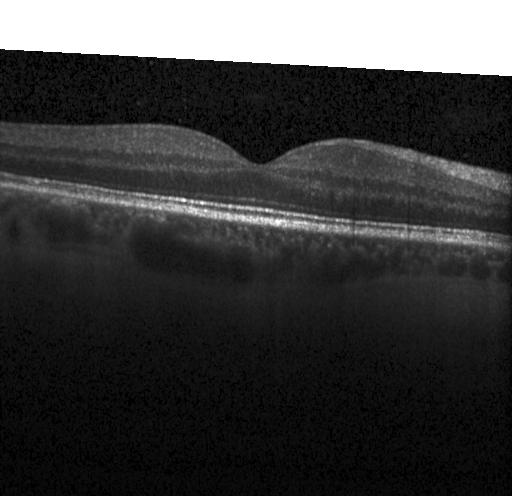

Optical coherence tomography scan; horizontal scan through the fovea; acquired on a Heidelberg Spectralis; spectral-domain optical coherence tomography. Impression: no evidence of CNV, DME, or drusen.